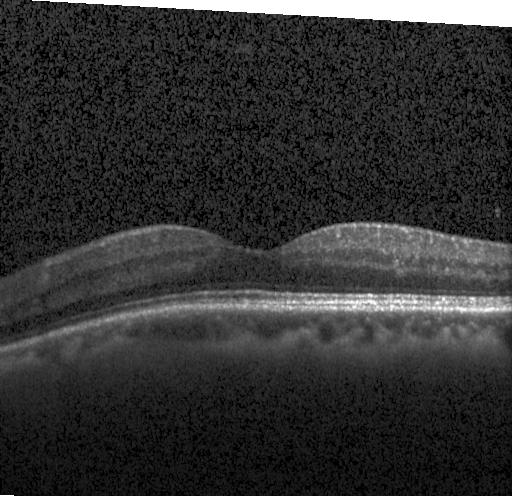

Heidelberg Spectralis. OCT line scan. Diagnosis: no CNV, no DME, and no drusen.